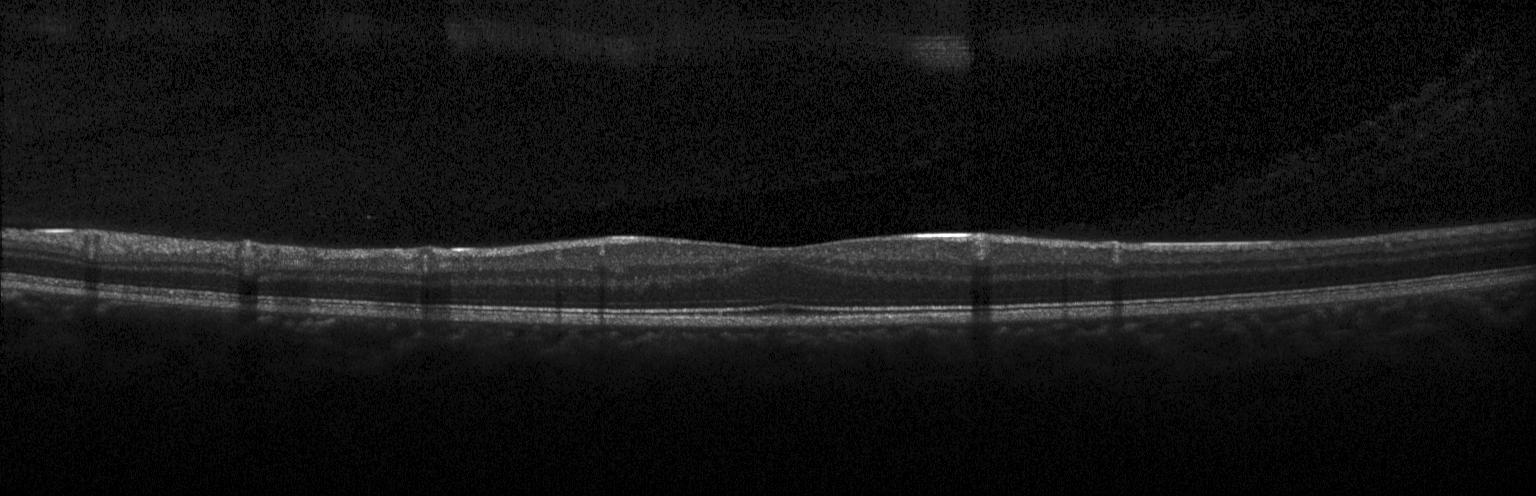

Heidelberg Spectralis OCT system · retinal OCT B-scan. OCT finding: neither choroidal neovascularization, diabetic macular edema, nor drusen.